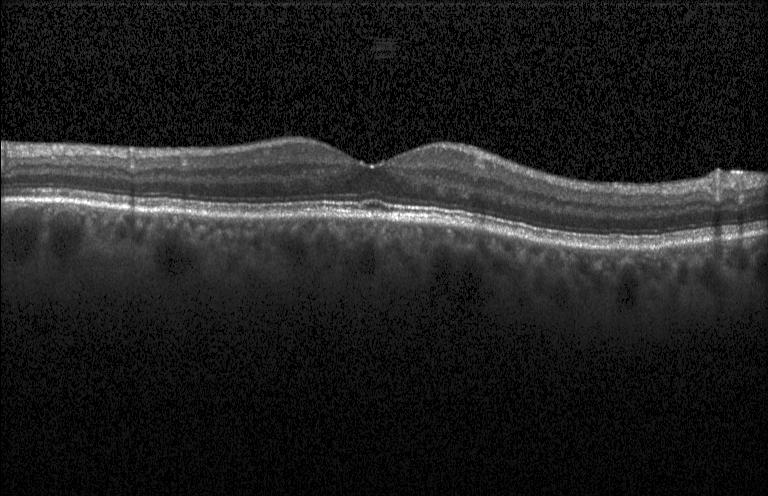
Optical coherence tomography B-scan. Acquired on a Heidelberg Spectralis. Centered on the fovea
Finding: no choroidal neovascularization, no diabetic macular edema, and no drusen.